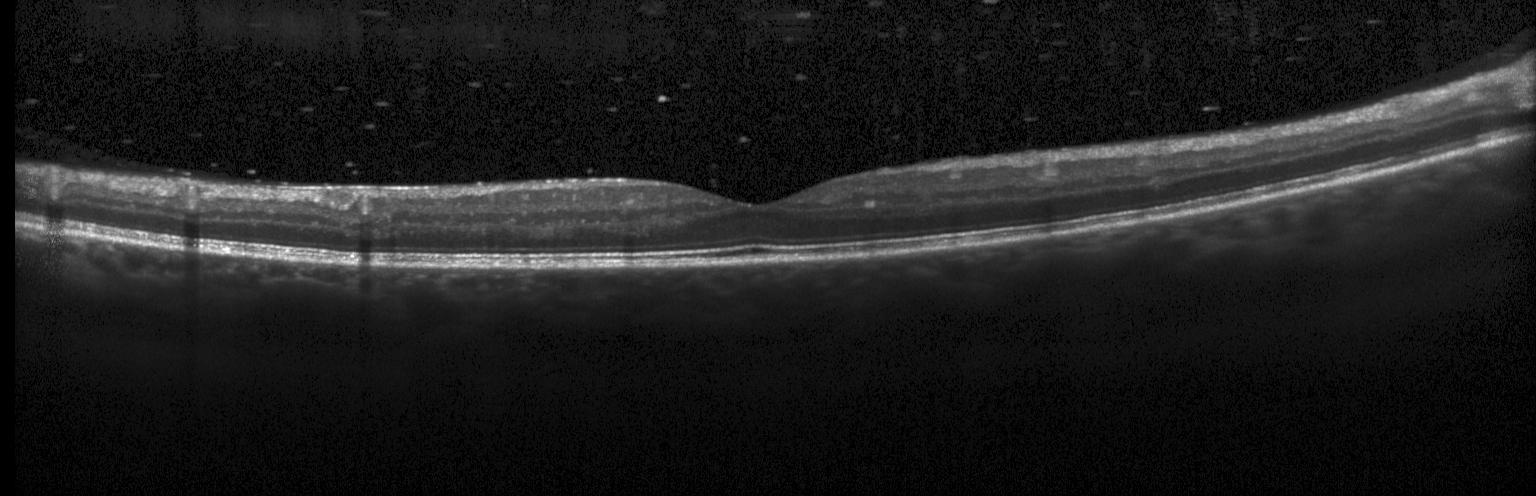
SD-OCT, OCT B-scan
Finding: neither choroidal neovascularization, diabetic macular edema, nor drusen.